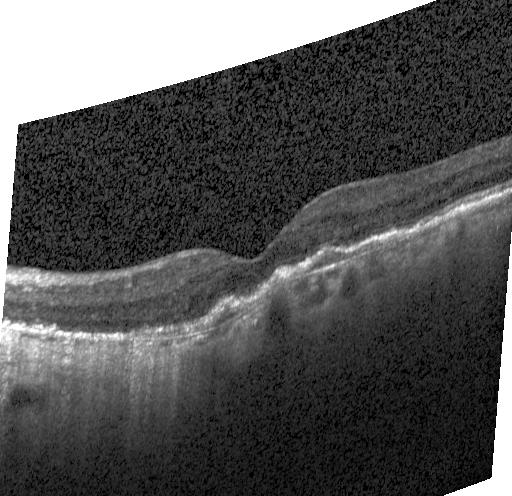

A choroidal neovascular membrane.